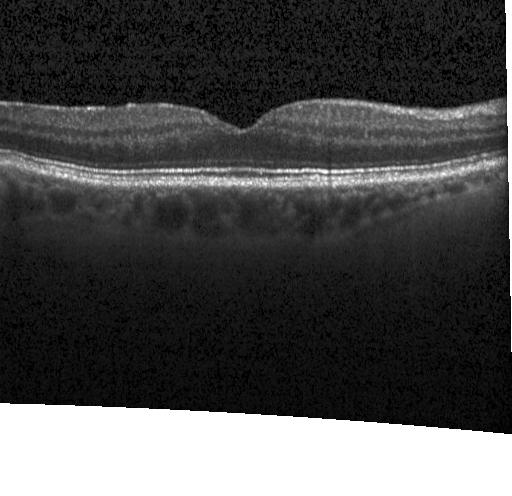 Acquired on a Heidelberg Spectralis. Retinal OCT cross-section. SD-OCT
Impression: neither CNV, DME, nor drusen.